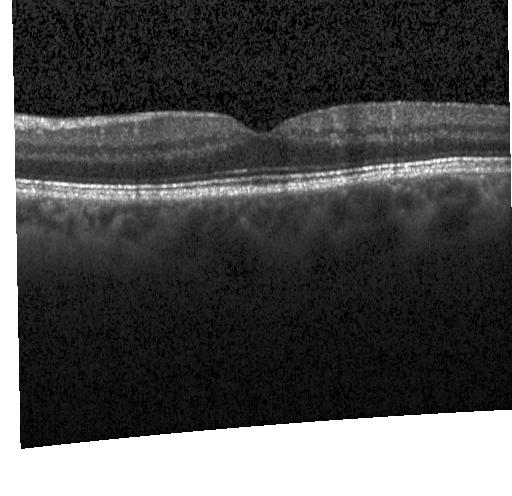
Retinal OCT B-scan.
This B-scan demonstrates no evidence of CNV, DME, or drusen.